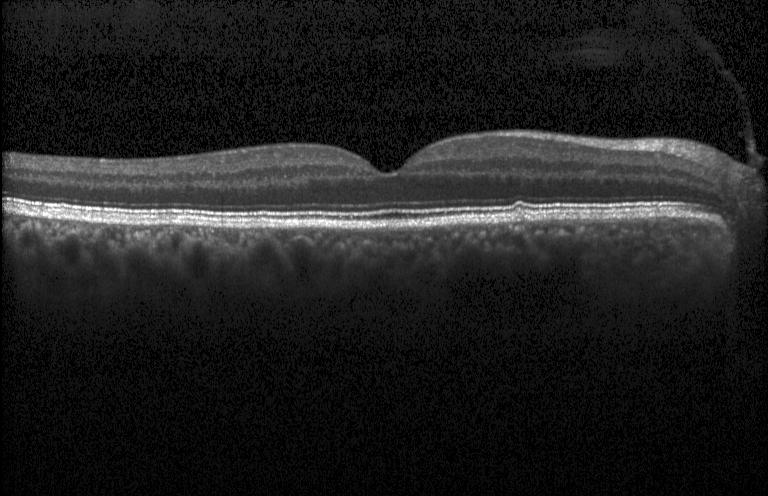
Finding: no evidence of choroidal neovascularization, diabetic macular edema, or drusen.